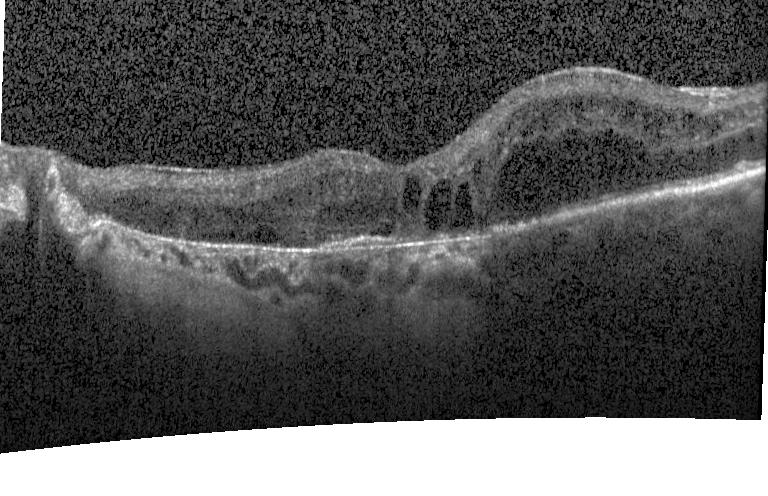 This B-scan demonstrates choroidal neovascularization.